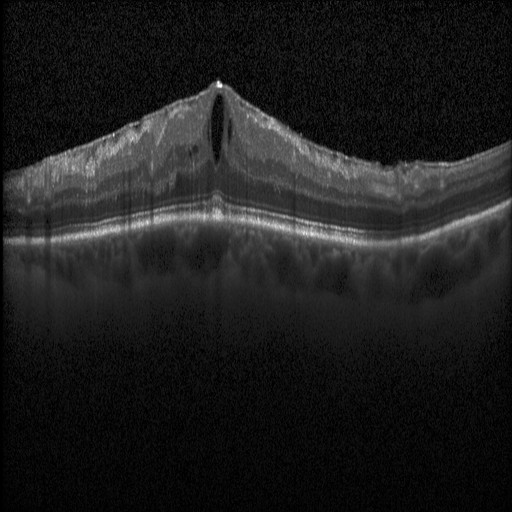
Assessment: diabetic macular edema.